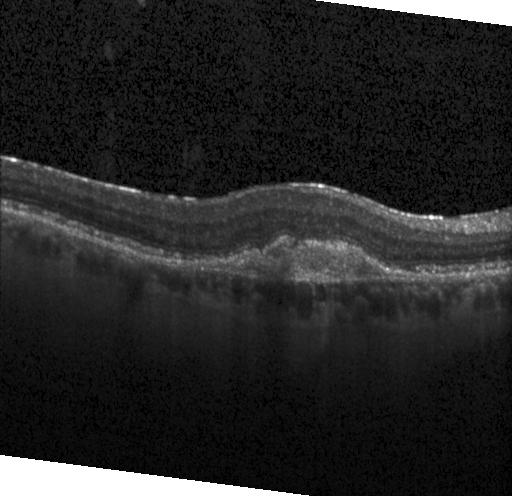

Macular OCT demonstrating CNV.